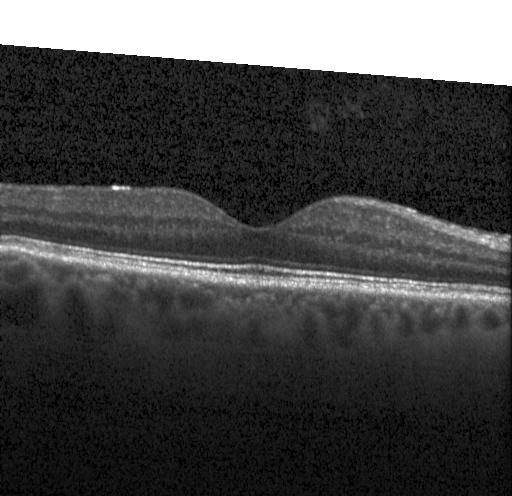
SD-OCT. Heidelberg Spectralis OCT system. Optical coherence tomography scan
This B-scan demonstrates no choroidal neovascularization, no diabetic macular edema, and no drusen.